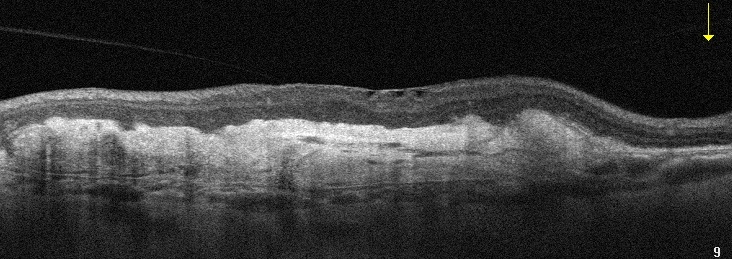

OCT scan showing age-related macular degeneration.